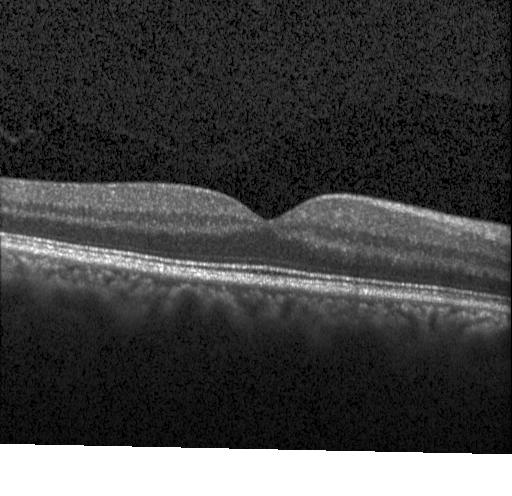 OCT B-scan showing no CNV, no DME, and no drusen.